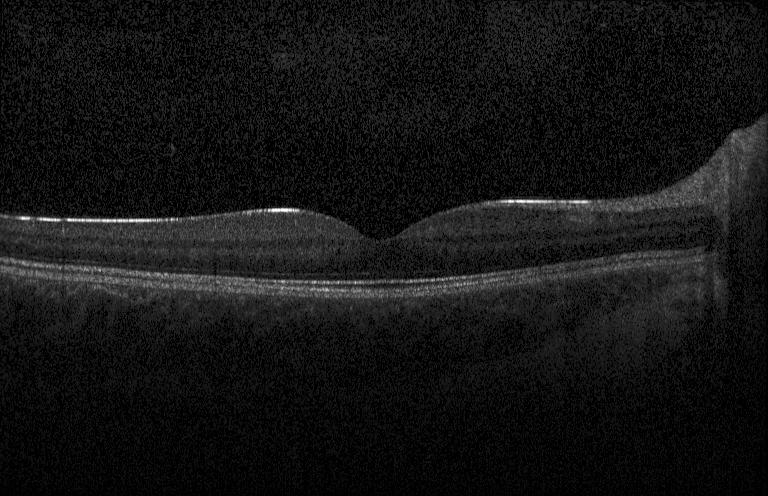 OCT B-scan. The scan shows no choroidal neovascularization, no diabetic macular edema, and no drusen.